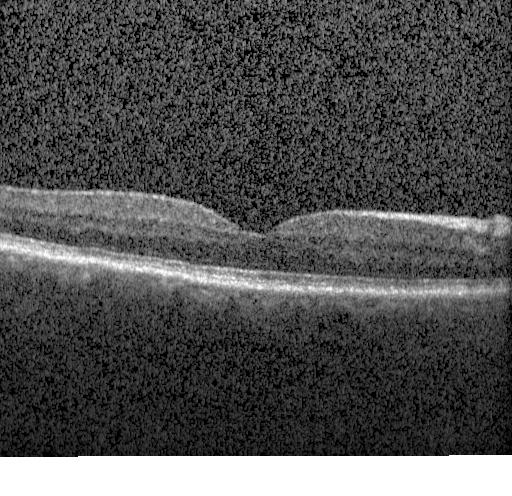
The scan shows neither choroidal neovascularization, diabetic macular edema, nor drusen.